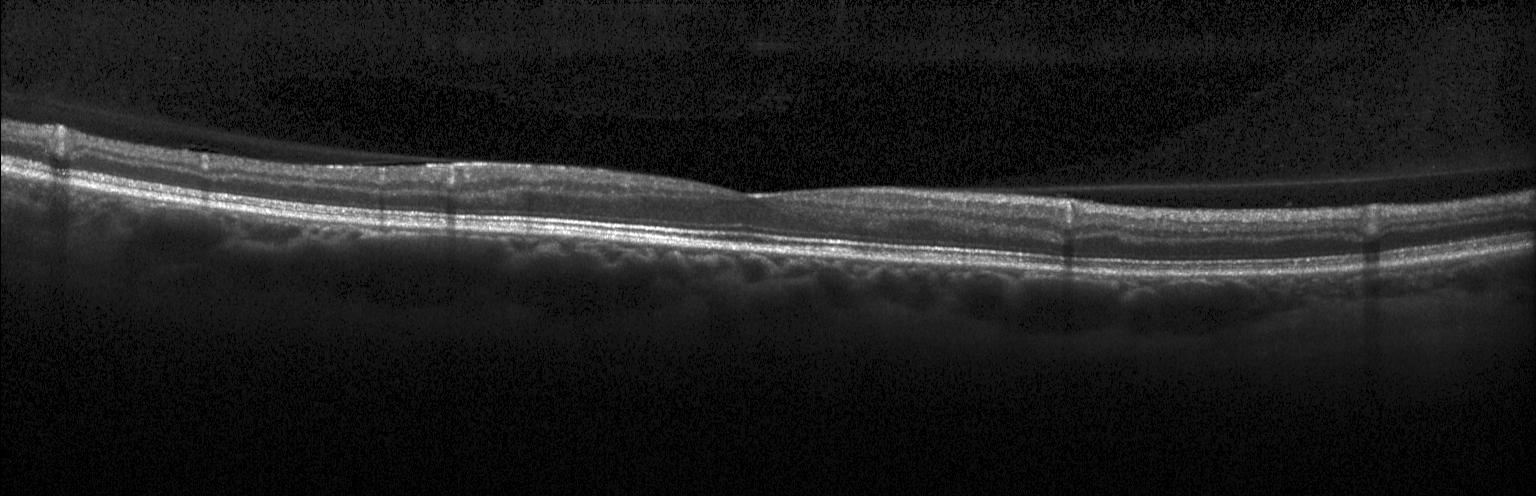
Impression: no CNV, DME, or drusen.